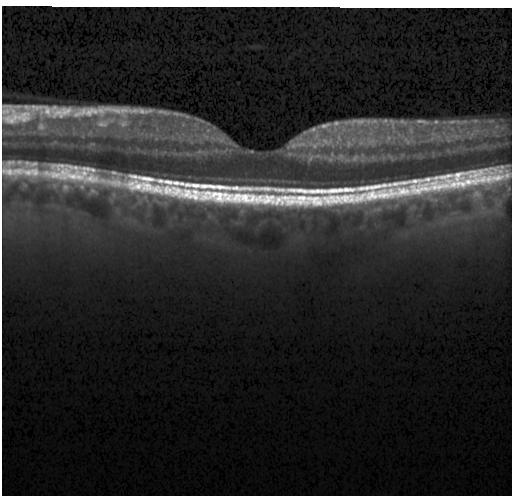
Diagnosis: neither choroidal neovascularization, diabetic macular edema, nor drusen.